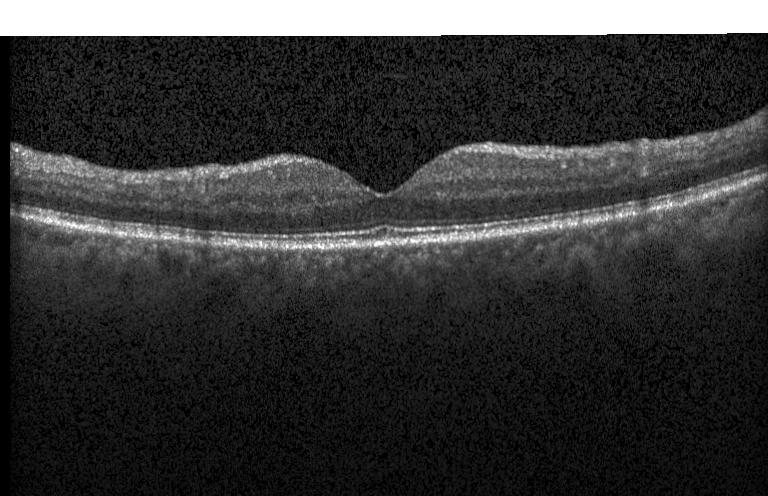

OCT line scan · centered on the fovea · spectral-domain OCT · instrument: Heidelberg Spectralis. Finding: no evidence of choroidal neovascularization, diabetic macular edema, or drusen.